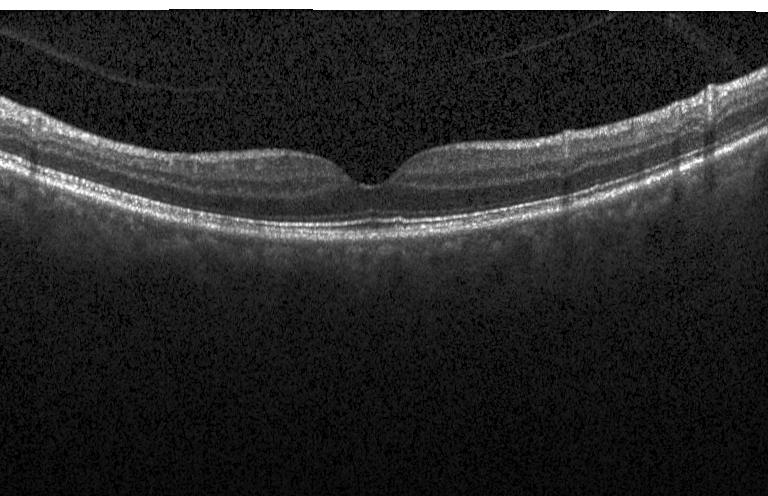
Heidelberg Spectralis OCT system; OCT line scan; SD-OCT; centered on the fovea — Finding: no CNV, no DME, and no drusen.